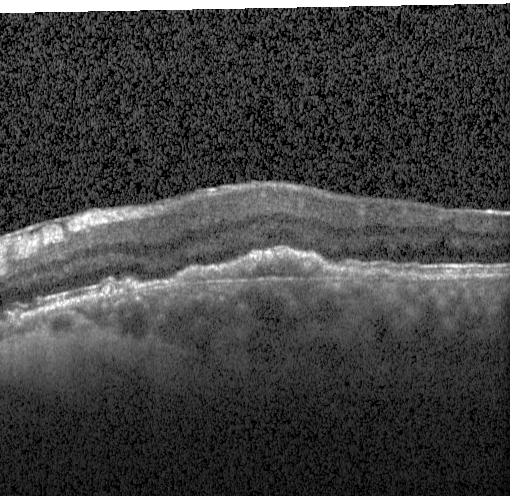
Finding: a choroidal neovascular membrane.